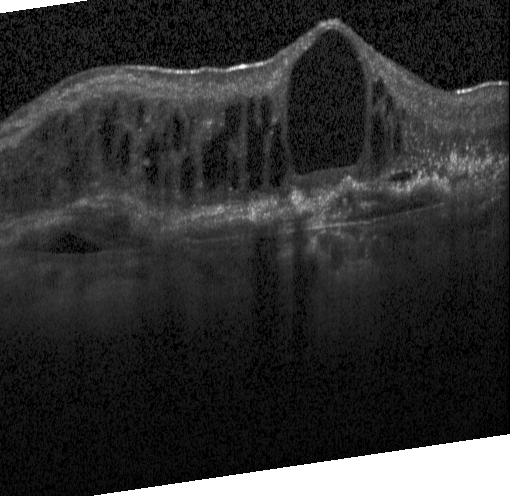
Spectral-domain OCT B-scan: a choroidal neovascular membrane.